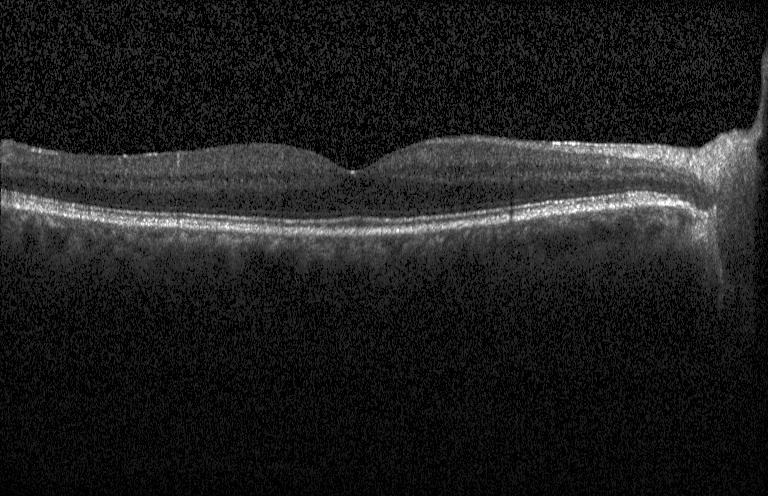

Optical coherence tomography B-scan · spectral-domain OCT · Heidelberg Spectralis OCT system · through the macula — Diagnosis: neither CNV, DME, nor drusen.